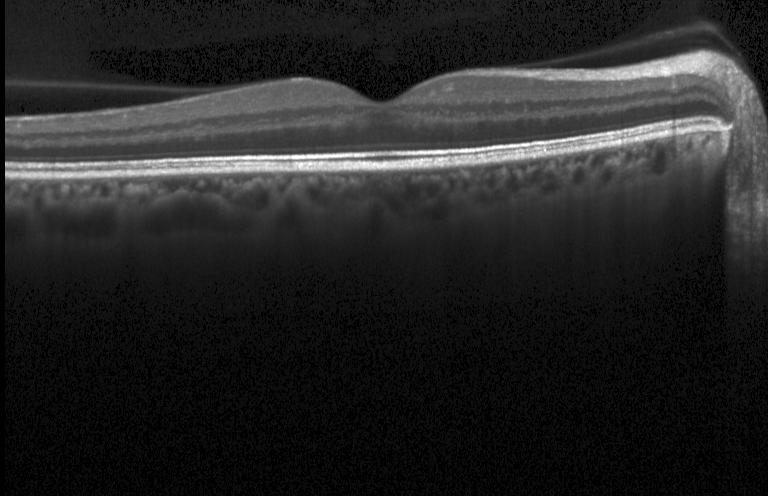 SD-OCT · OCT line scan
Macular OCT: neither choroidal neovascularization, diabetic macular edema, nor drusen.